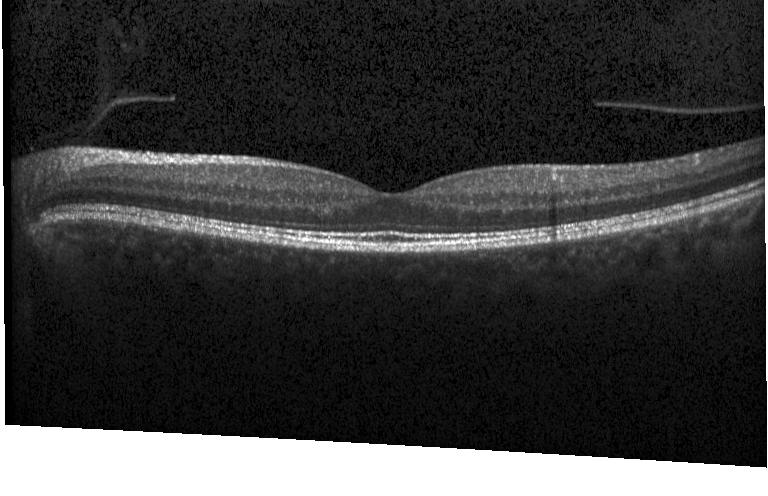 Retinal OCT cross-section. Impression: no choroidal neovascularization, diabetic macular edema, or drusen.